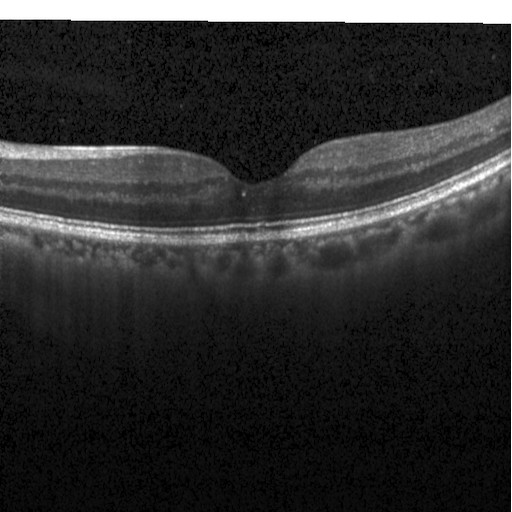 Optical coherence tomography B-scan. Spectral-domain optical coherence tomography. Instrument: Heidelberg Spectralis
Macular OCT: diabetic macular edema (DME).